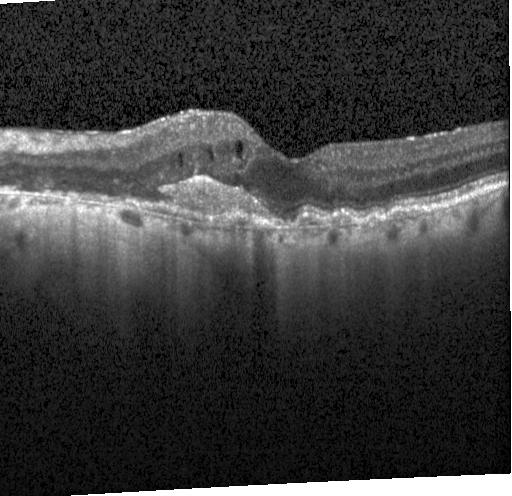

Fovea-centered; retinal OCT cross-section; Heidelberg Spectralis
Assessment: a choroidal neovascular membrane.